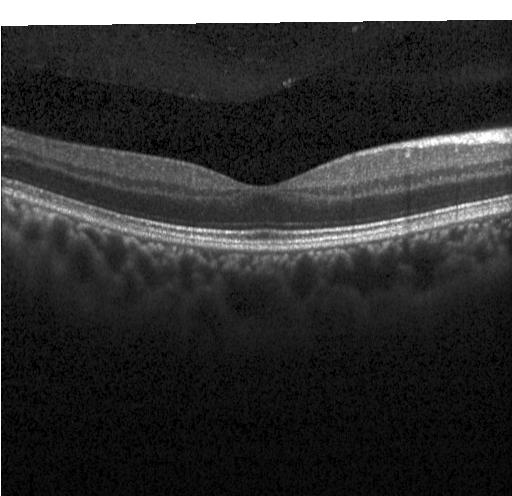 This B-scan demonstrates neither CNV, DME, nor drusen.